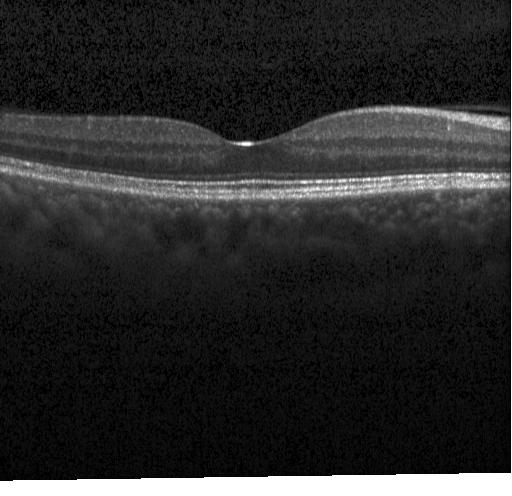 Optical coherence tomography B-scan, instrument: Heidelberg Spectralis — Assessment: no choroidal neovascularization, no diabetic macular edema, and no drusen.